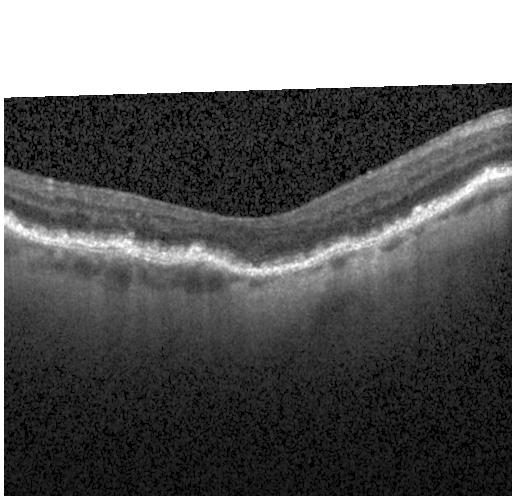

Optical coherence tomography B-scan; spectral-domain OCT. Diagnosis: choroidal neovascularization (CNV).